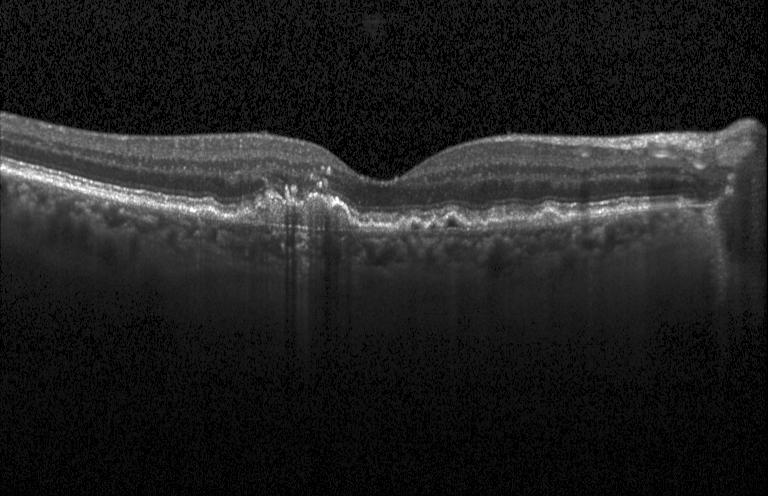

Optical coherence tomography scan. Heidelberg Spectralis OCT system. Spectral-domain OCT. Centered on the fovea
Macular OCT: a choroidal neovascular membrane.